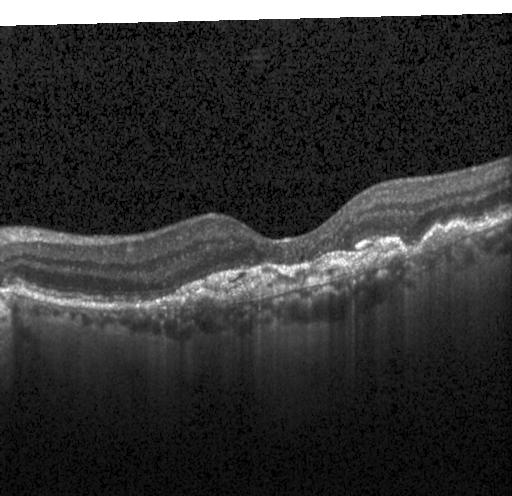
Retinal OCT cross-section. Diagnosis: a choroidal neovascular membrane.